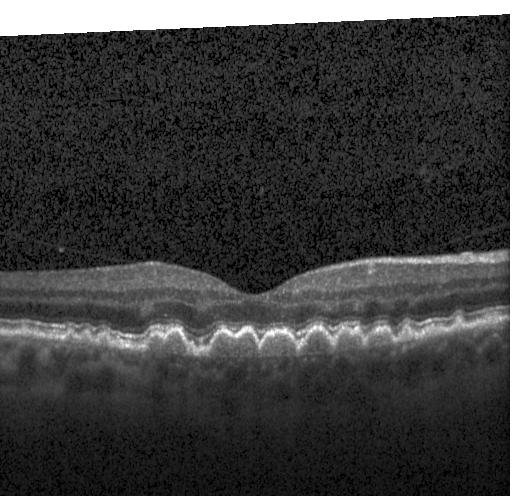

Drusen.